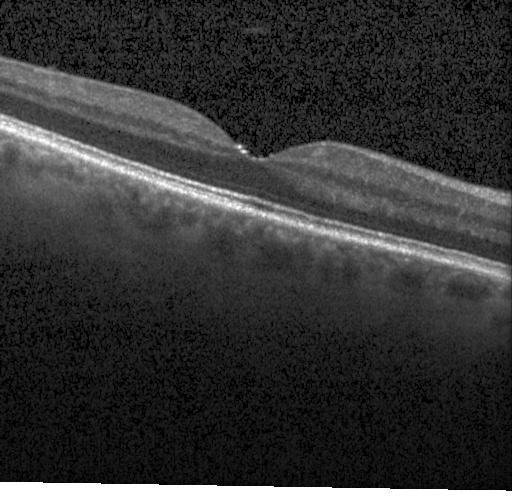

Diagnosis: no CNV, DME, or drusen.